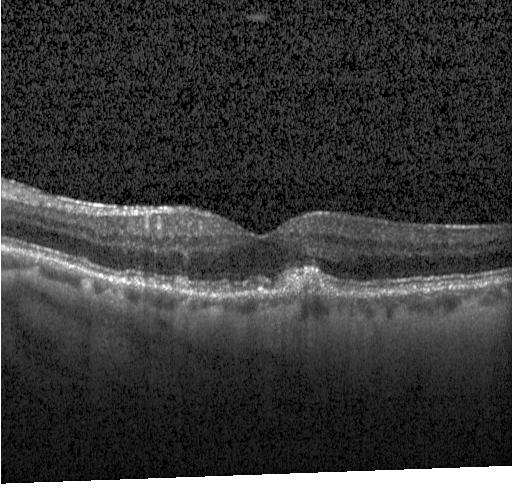

Retinal OCT B-scan, acquired on a Heidelberg Spectralis — Sub-RPE drusenoid deposits.